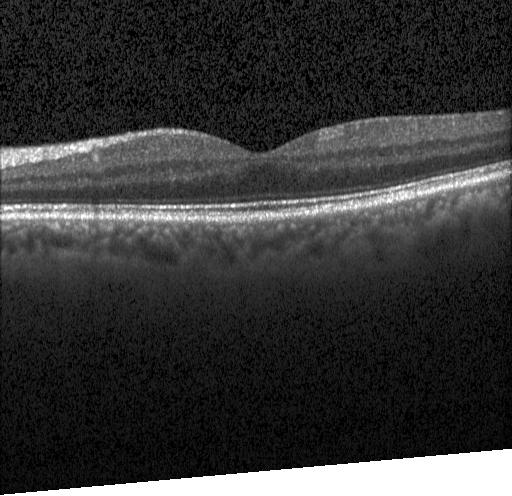 Macular OCT demonstrating neither choroidal neovascularization, diabetic macular edema, nor drusen.